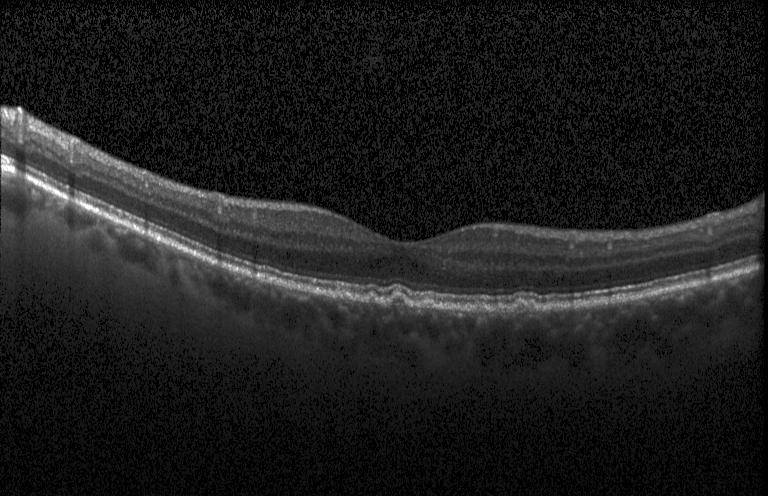

Finding: multiple drusen.